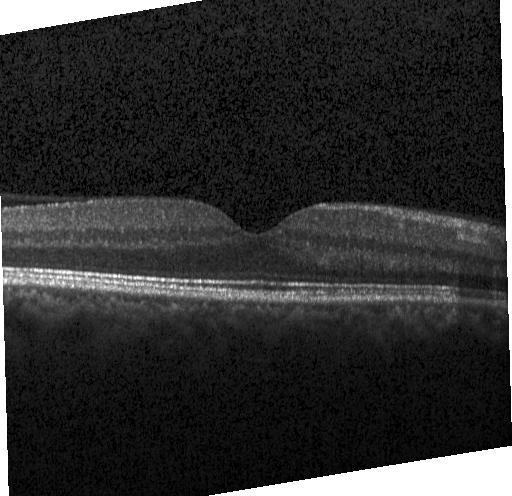
Through the macula; retinal OCT cross-section; Heidelberg Spectralis — Finding: no evidence of choroidal neovascularization, diabetic macular edema, or drusen.